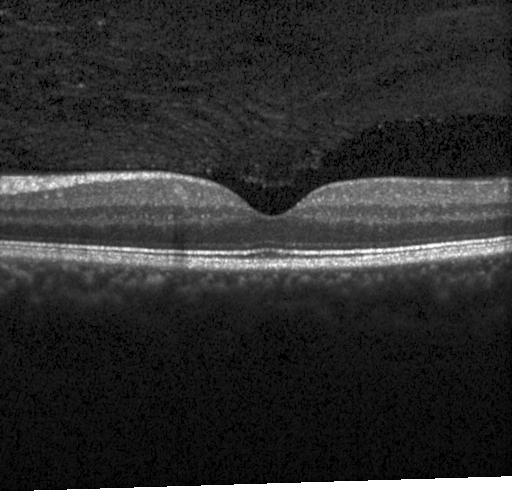
Macular scan. Heidelberg Spectralis OCT system. OCT B-scan
Dx: no choroidal neovascularization, diabetic macular edema, or drusen.